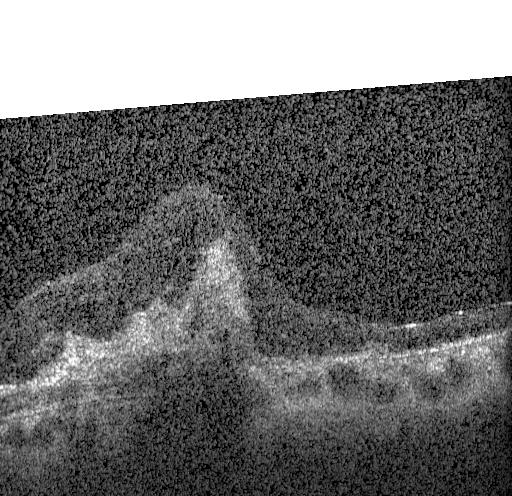 Instrument: Heidelberg Spectralis. OCT line scan. SD-OCT — Assessment: a choroidal neovascular membrane.